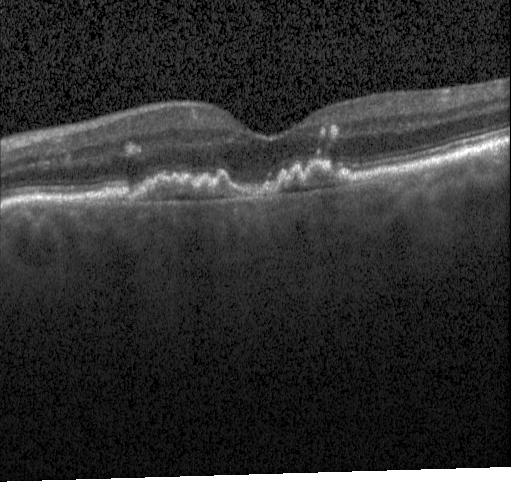
SD-OCT · acquired on a Heidelberg Spectralis · retinal OCT cross-section
Assessment: a choroidal neovascular membrane.